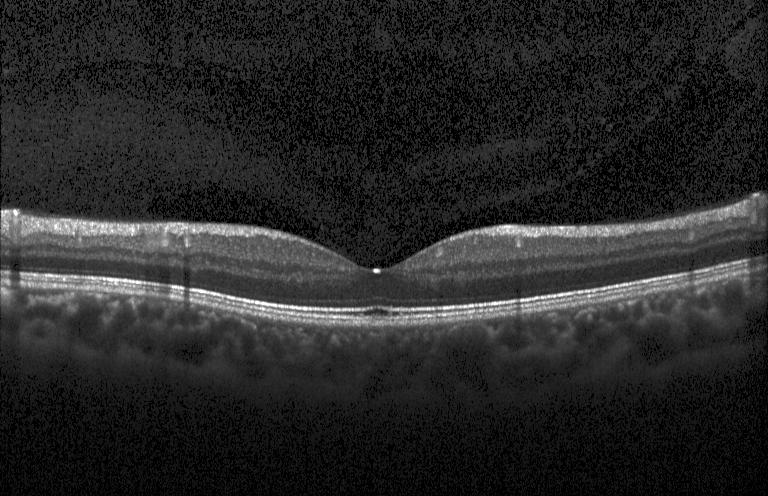 OCT finding: no evidence of choroidal neovascularization, diabetic macular edema, or drusen.